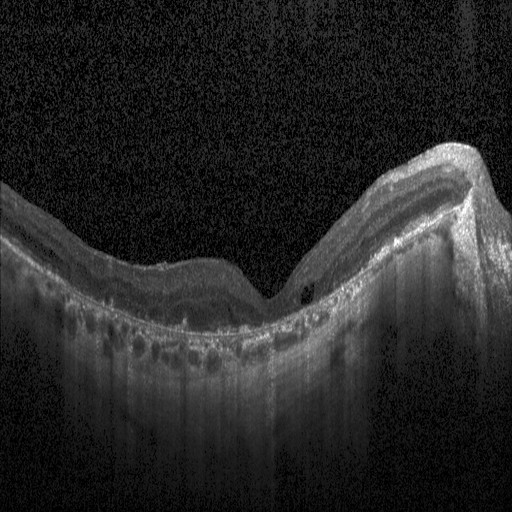
Fovea-centered. Heidelberg Spectralis. Retinal OCT B-scan. Impression: DME.